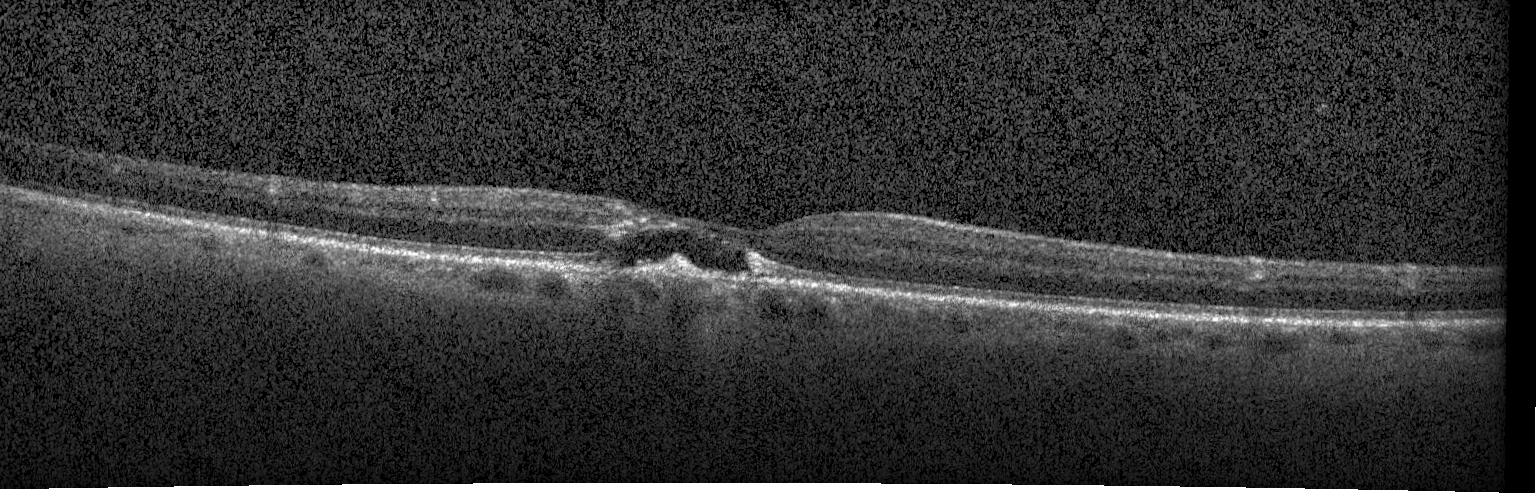

Retinal OCT B-scan. Diagnosis: CNV.